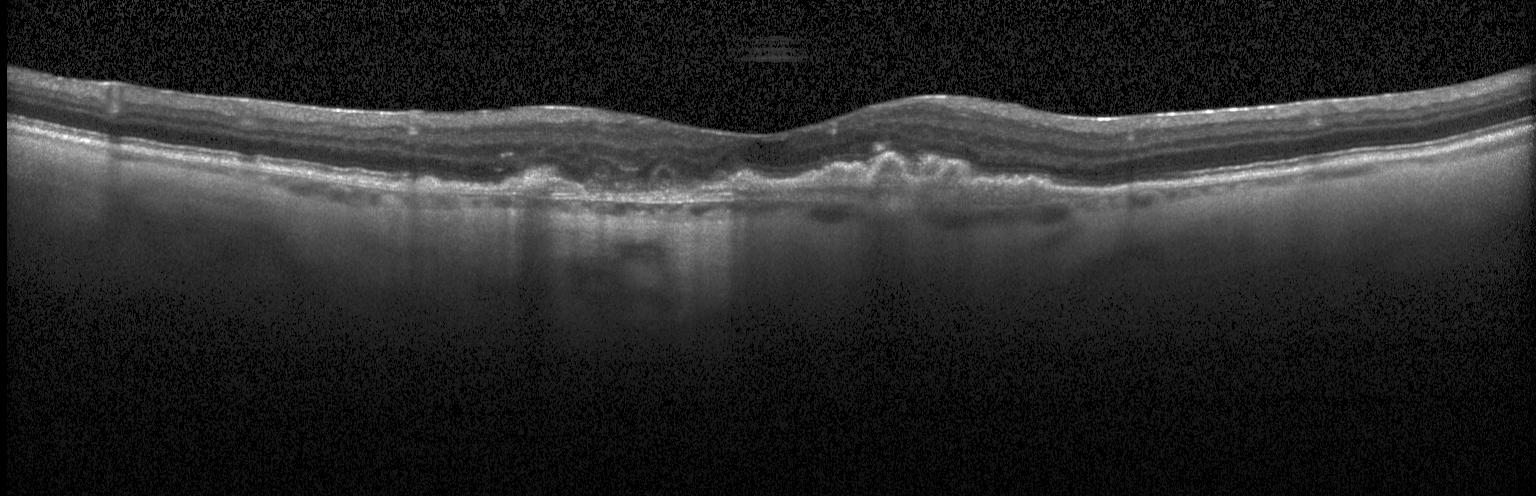
Spectral-domain OCT, retinal OCT B-scan. Dx: a choroidal neovascular membrane.